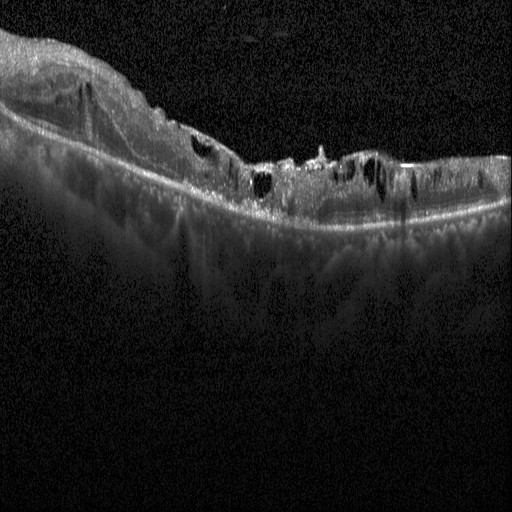

Dx: diabetic macular edema.